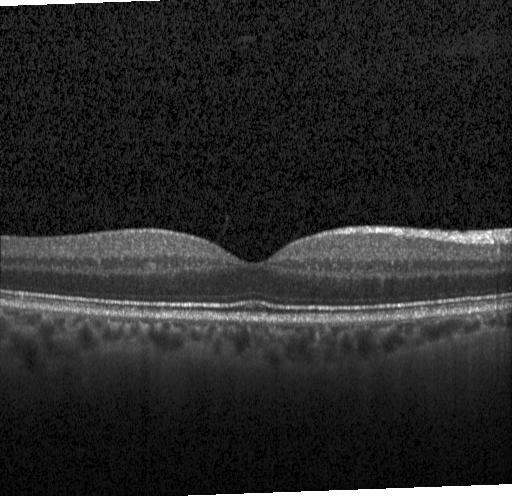

Dx: no evidence of CNV, DME, or drusen.